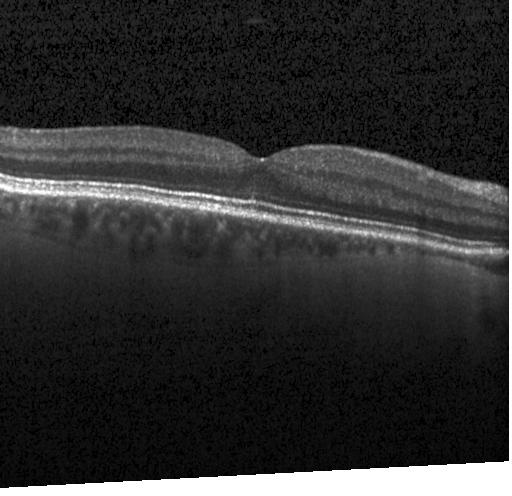

Instrument: Heidelberg Spectralis; centered on the fovea; SD-OCT; optical coherence tomography scan
OCT finding: neither CNV, DME, nor drusen.